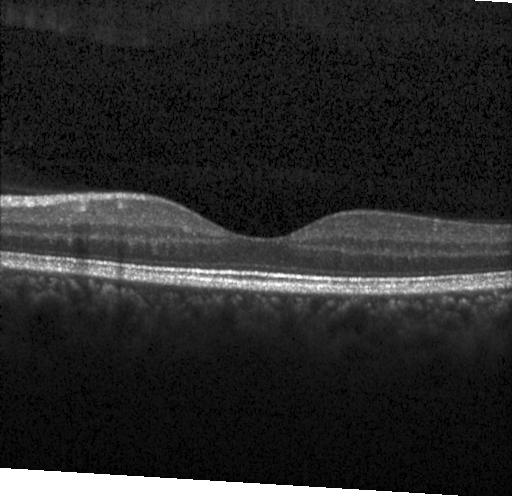 Spectral-domain OCT. Optical coherence tomography B-scan. Instrument: Heidelberg Spectralis — Dx: no CNV, DME, or drusen.